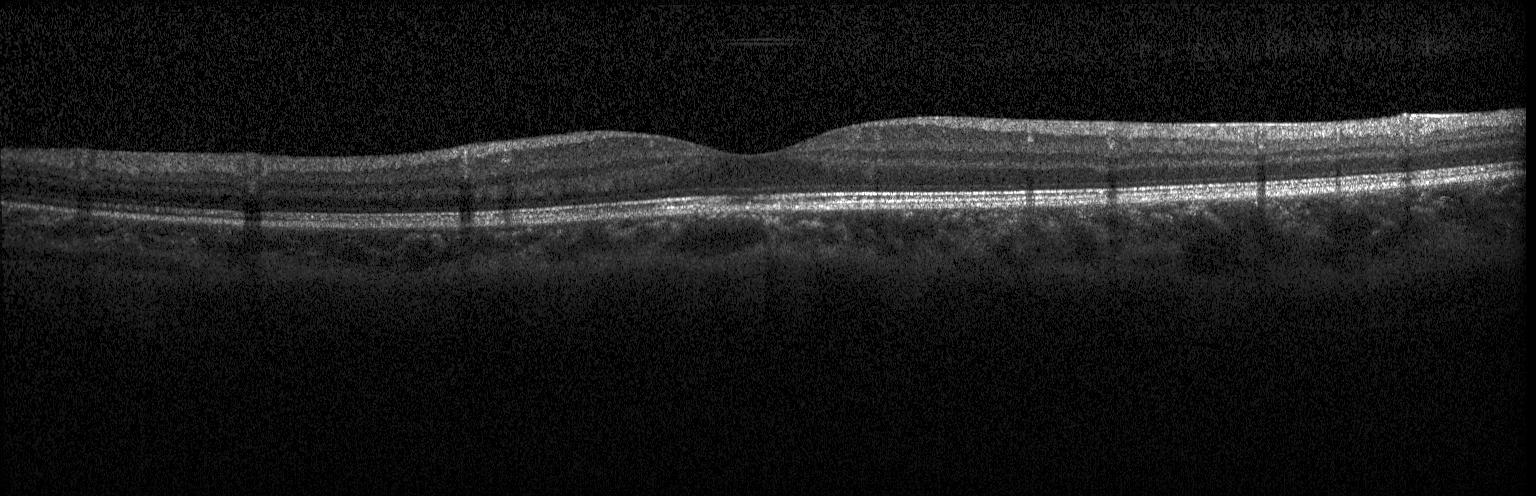

Centered on the fovea; SD-OCT; optical coherence tomography B-scan — The scan shows neither choroidal neovascularization, diabetic macular edema, nor drusen.